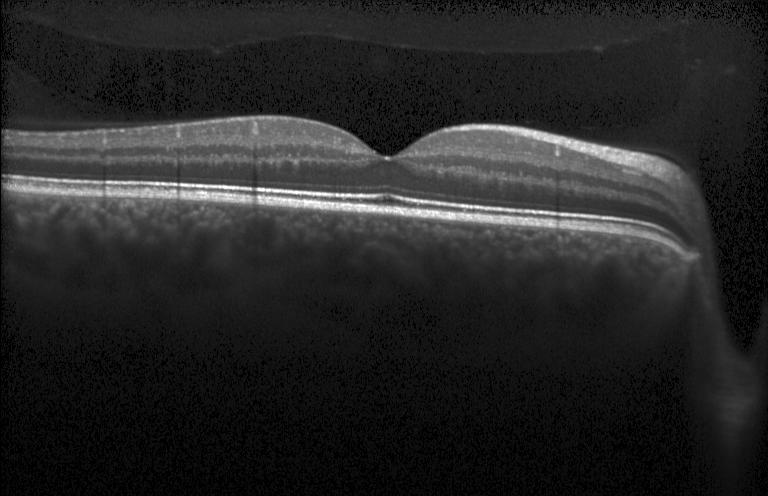
Spectral-domain optical coherence tomography. OCT B-scan. Assessment: no CNV, no DME, and no drusen.